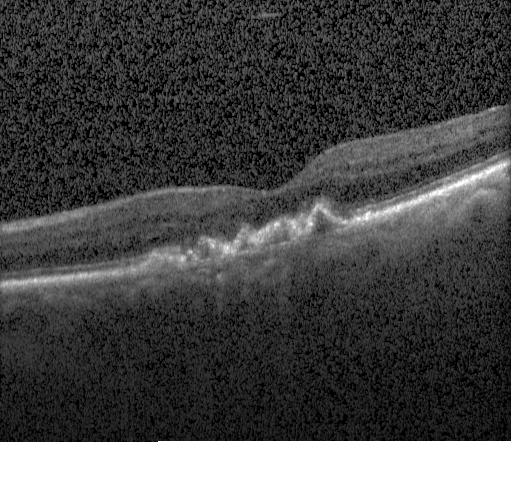

Assessment: sub-RPE drusenoid deposits.